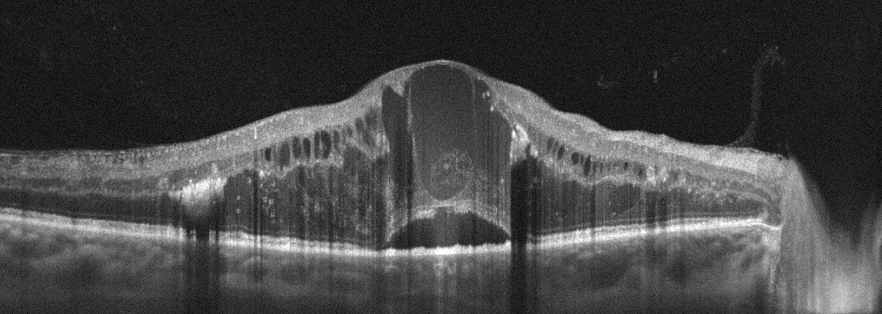 Impression: RVO.